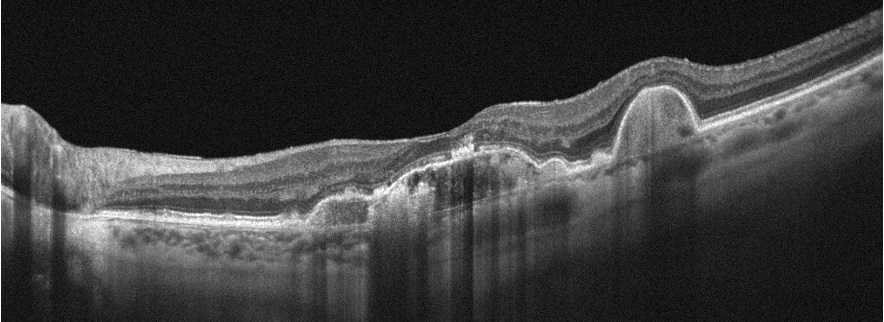
Impression: age-related macular degeneration (AMD).